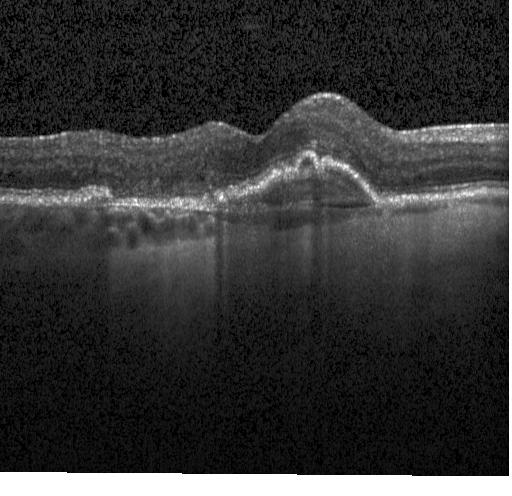
Retinal OCT B-scan · horizontal scan through the fovea · Heidelberg Spectralis · spectral-domain optical coherence tomography
The scan shows a choroidal neovascular membrane.